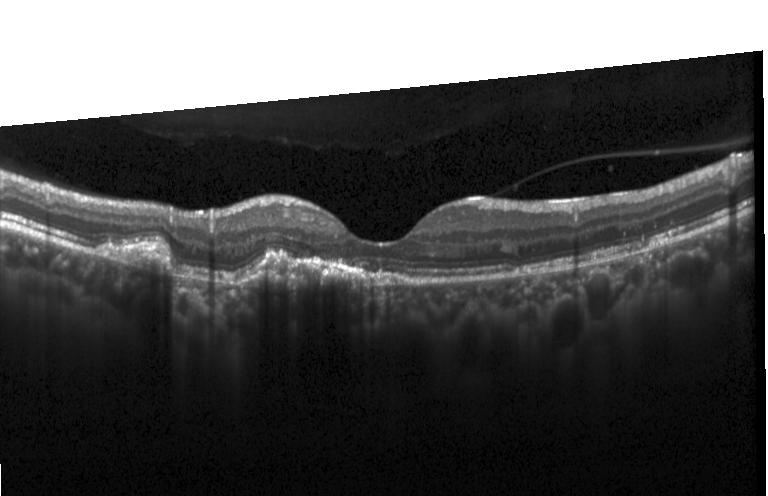
Optical coherence tomography scan — A choroidal neovascular membrane.